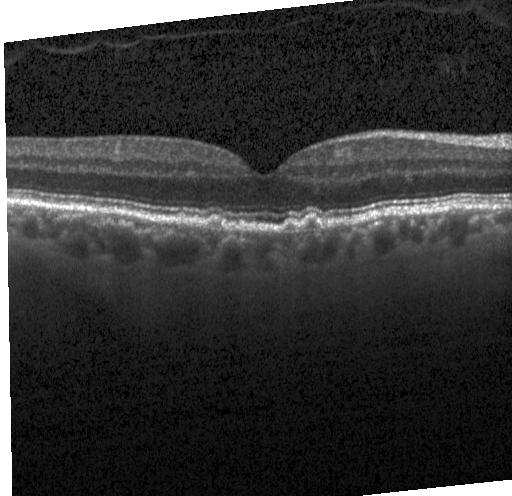
Dx: sub-RPE drusenoid deposits.